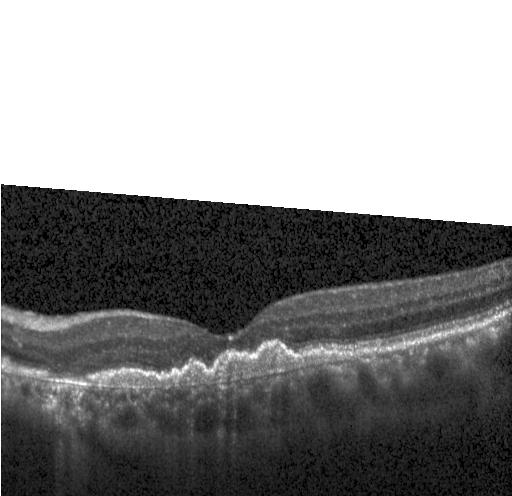
This B-scan demonstrates choroidal neovascularization.